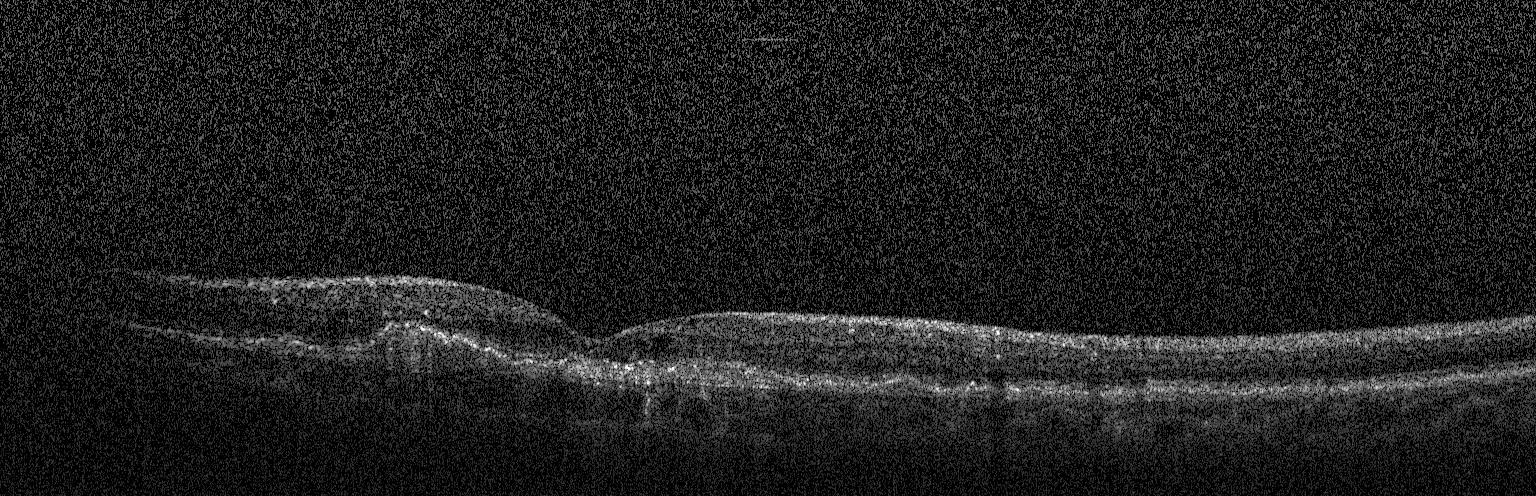 Optical coherence tomography scan. Diagnosis: a choroidal neovascular membrane.